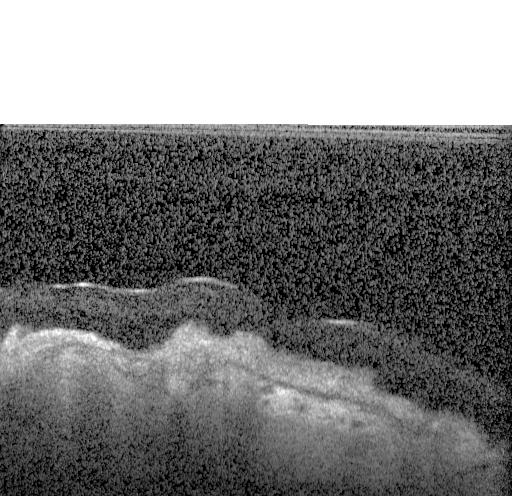

OCT line scan.
Dx: a choroidal neovascular membrane.